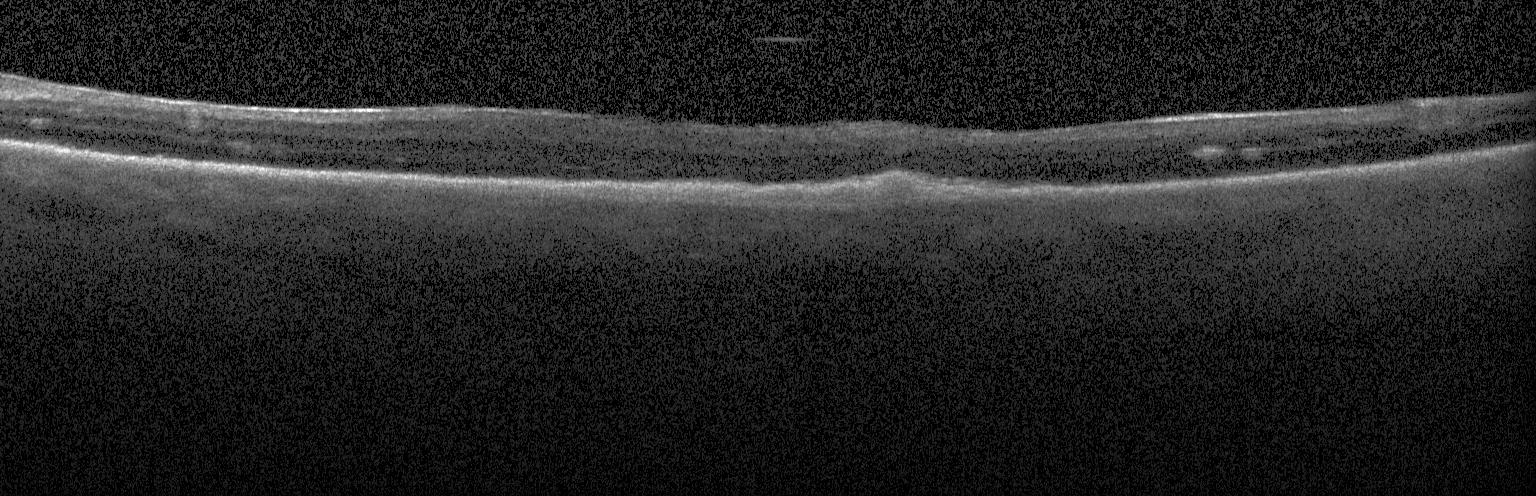

SD-OCT; macular scan; Heidelberg Spectralis OCT system; retinal OCT B-scan. Diagnosis: a choroidal neovascular membrane.